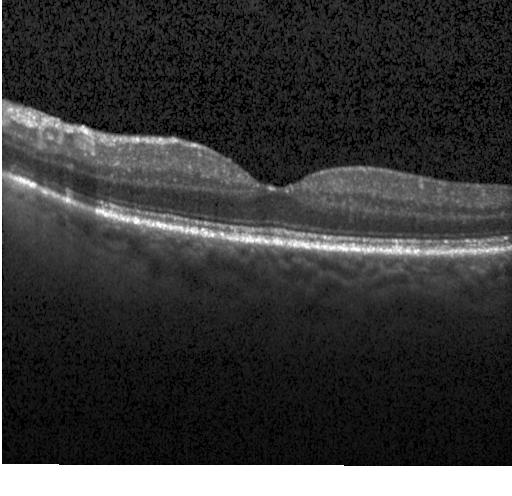 Macular OCT demonstrating no CNV, DME, or drusen.